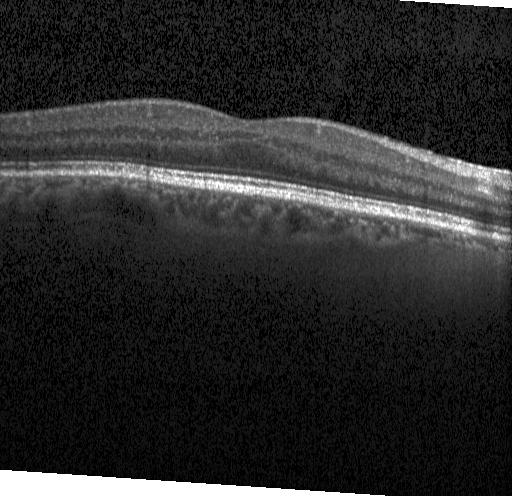 Instrument: Heidelberg Spectralis, retinal OCT cross-section — Impression: no choroidal neovascularization, diabetic macular edema, or drusen.